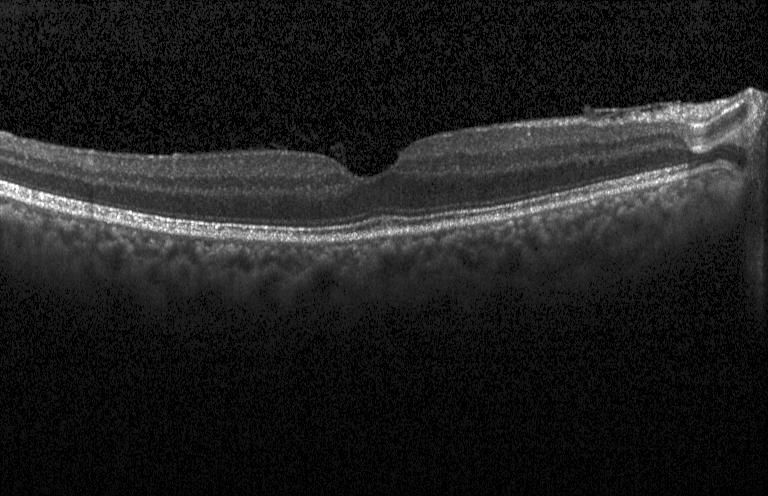

OCT scan showing no CNV, no DME, and no drusen.